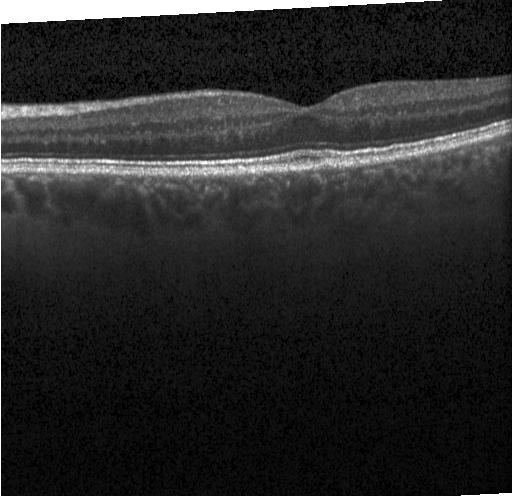
Macular OCT demonstrating neither choroidal neovascularization, diabetic macular edema, nor drusen.